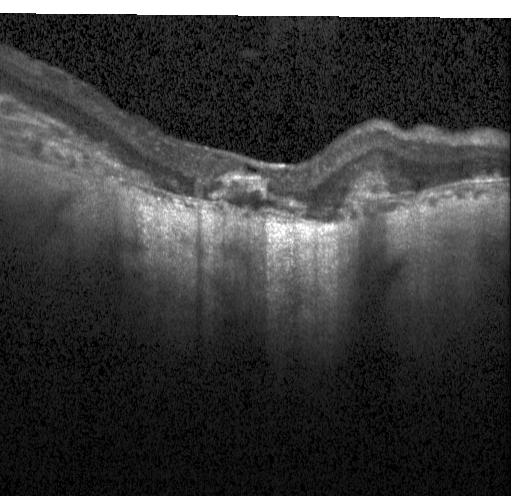 Retinal OCT cross-section showing choroidal neovascularization (CNV).